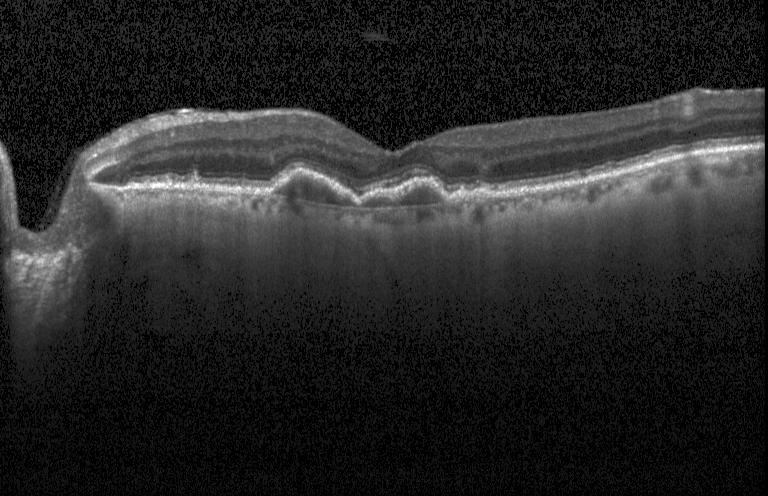 Retinal OCT cross-section — Impression: a choroidal neovascular membrane.